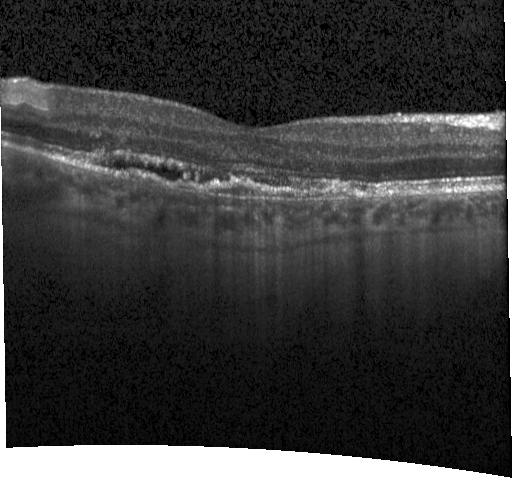 Optical coherence tomography scan
Diagnosis: a choroidal neovascular membrane.